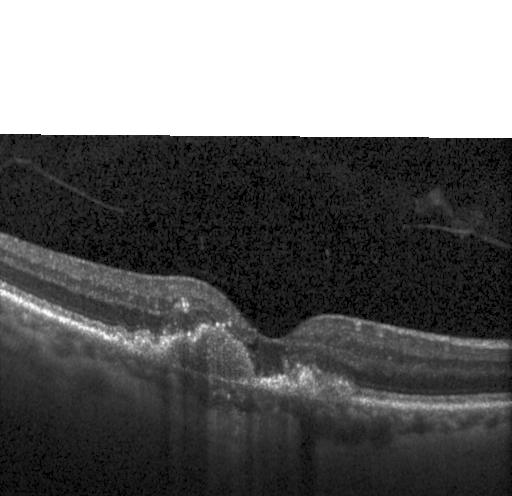 Instrument: Heidelberg Spectralis. Fovea-centered. Optical coherence tomography B-scan
This B-scan demonstrates a choroidal neovascular membrane.